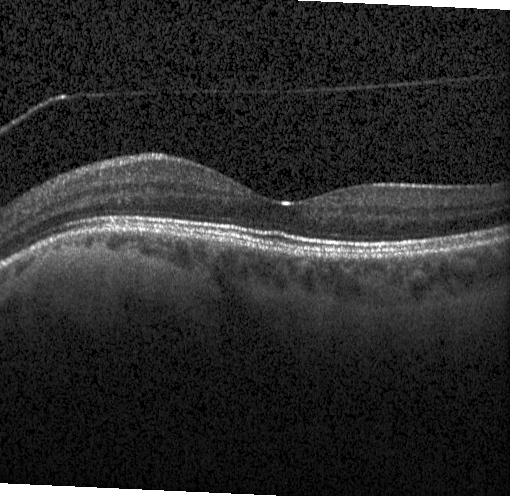 SD-OCT, OCT B-scan.
Impression: no CNV, DME, or drusen.